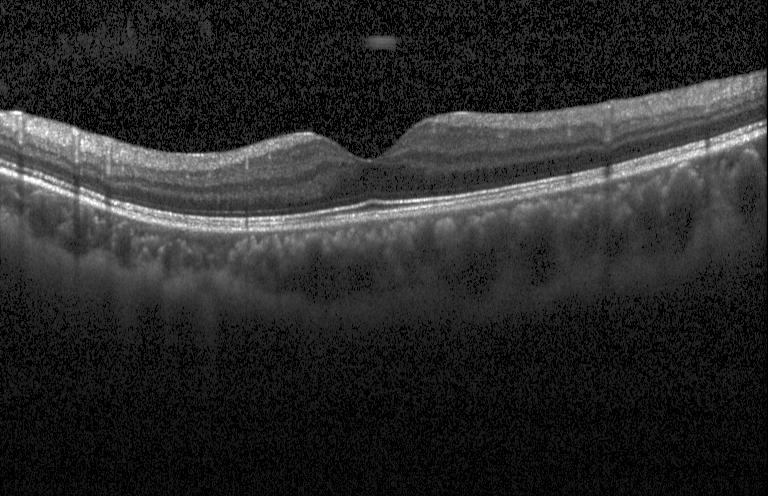
Through the macula, spectral-domain optical coherence tomography, retinal OCT cross-section
Impression: neither CNV, DME, nor drusen.